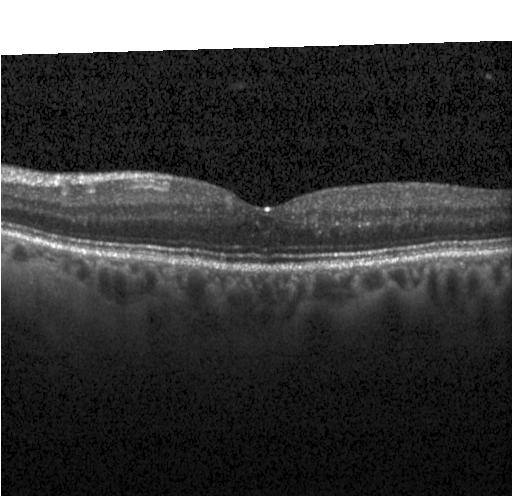

Spectral-domain OCT · instrument: Heidelberg Spectralis · OCT B-scan
The scan shows no choroidal neovascularization, diabetic macular edema, or drusen.